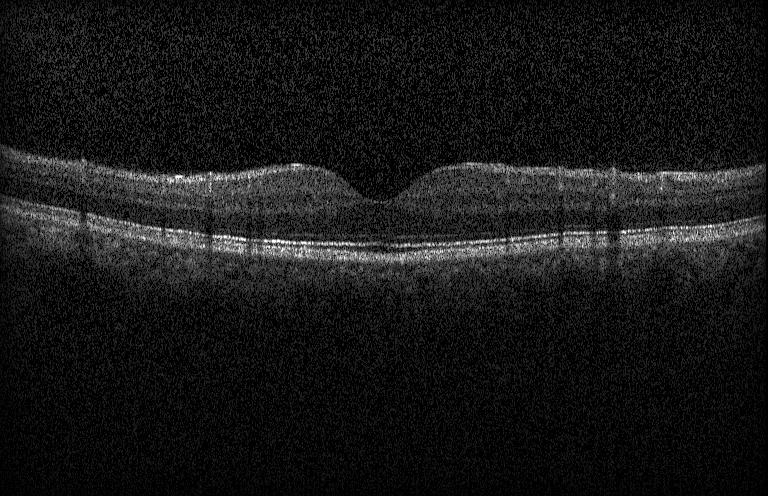
Spectral-domain optical coherence tomography; OCT line scan. This B-scan demonstrates no choroidal neovascularization, diabetic macular edema, or drusen.